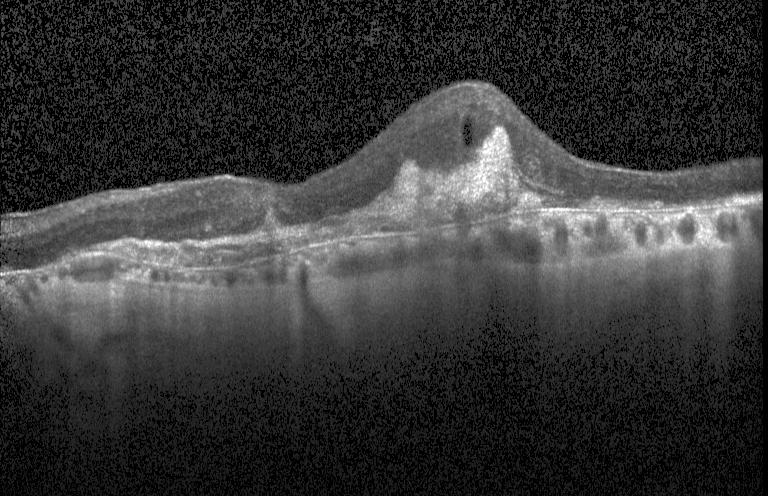

Impression: choroidal neovascularization.